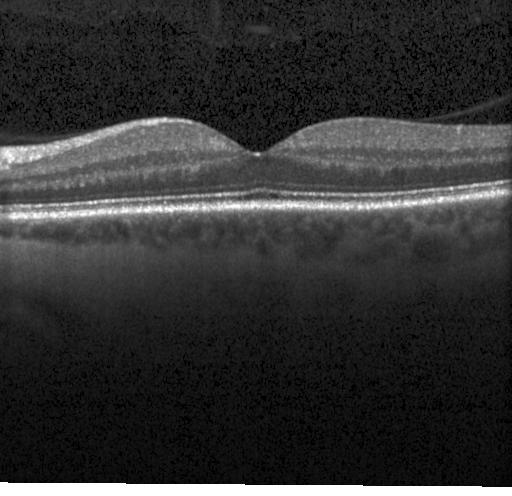 Impression: no CNV, DME, or drusen.